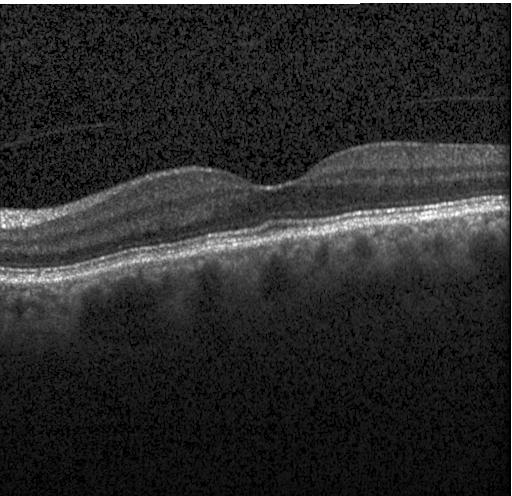 Retinal OCT cross-section · spectral-domain optical coherence tomography · macular scan — Diagnosis: no evidence of choroidal neovascularization, diabetic macular edema, or drusen.